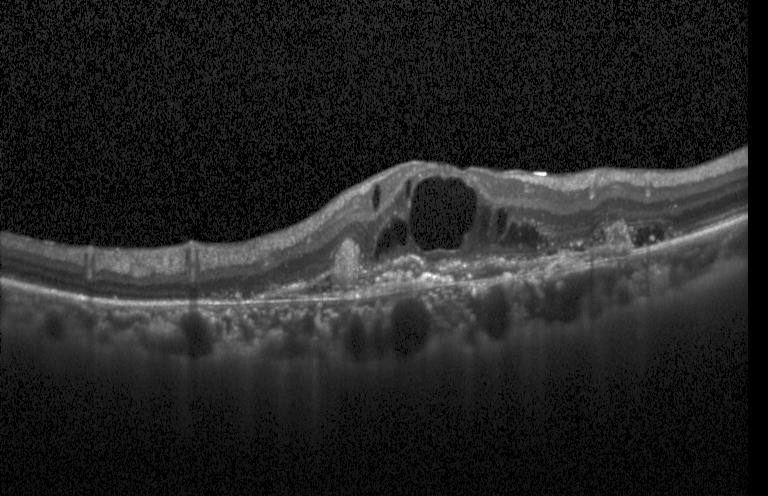 The scan shows a choroidal neovascular membrane.